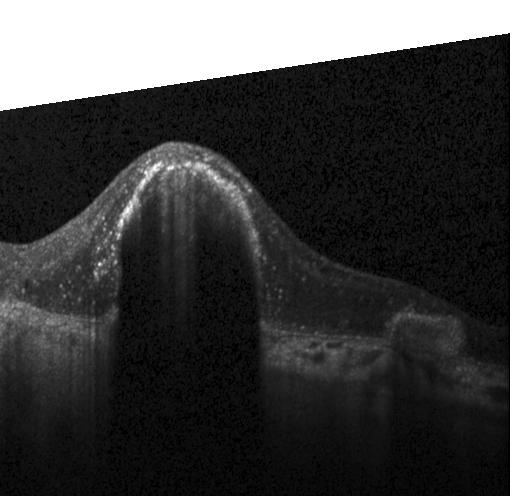 Diagnosis: choroidal neovascularization (CNV).